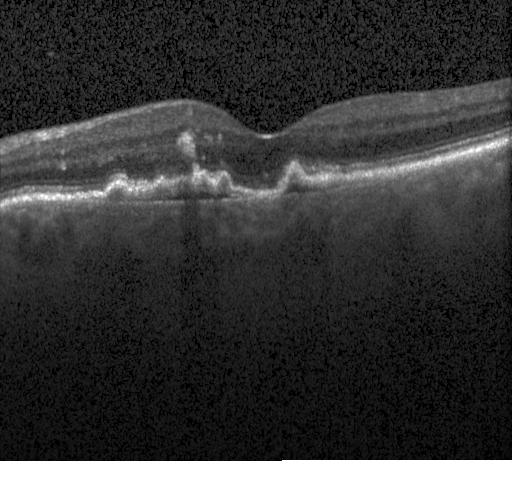
Diagnosis: choroidal neovascularization.